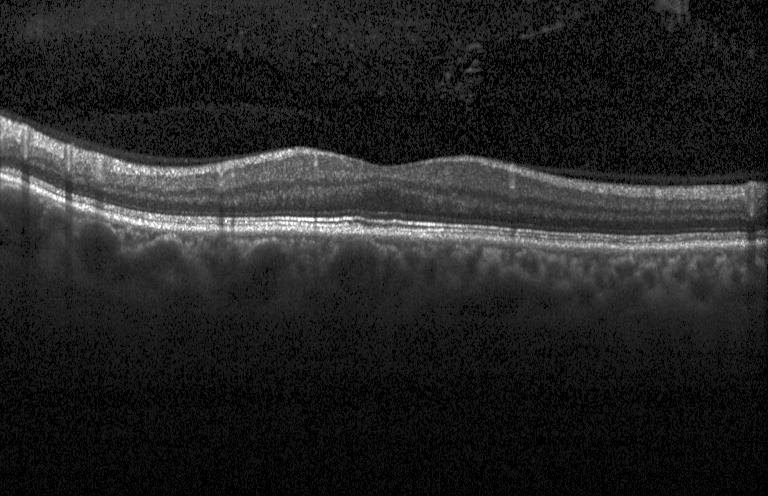 Optical coherence tomography scan.
Impression: no choroidal neovascularization, diabetic macular edema, or drusen.